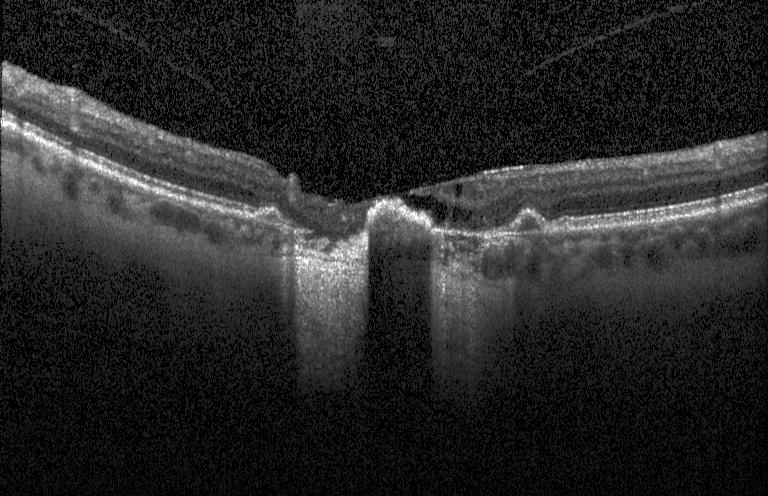 OCT scan showing a choroidal neovascular membrane.